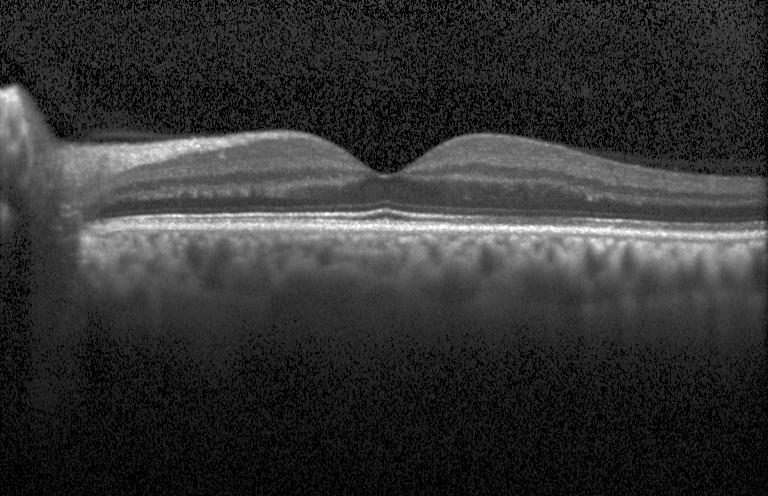 Diagnosis: no choroidal neovascularization, no diabetic macular edema, and no drusen.